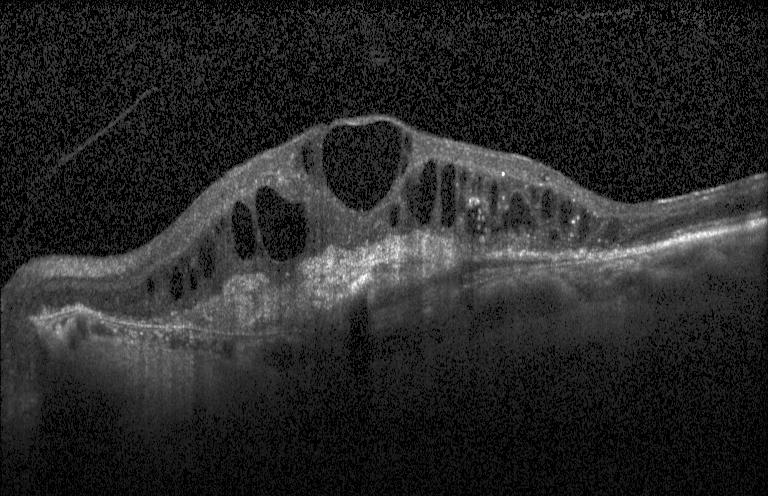

Diagnosis: choroidal neovascularization.